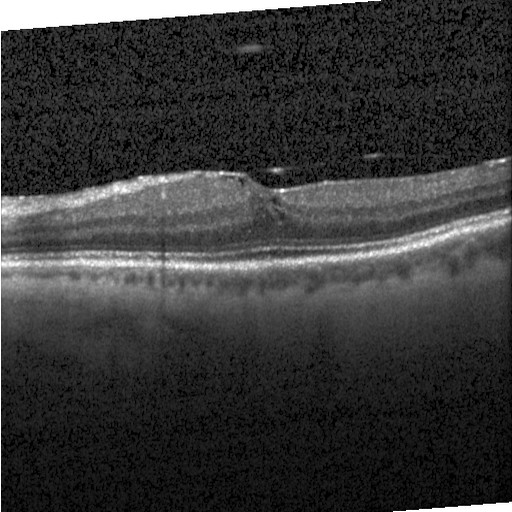
Finding: DME.